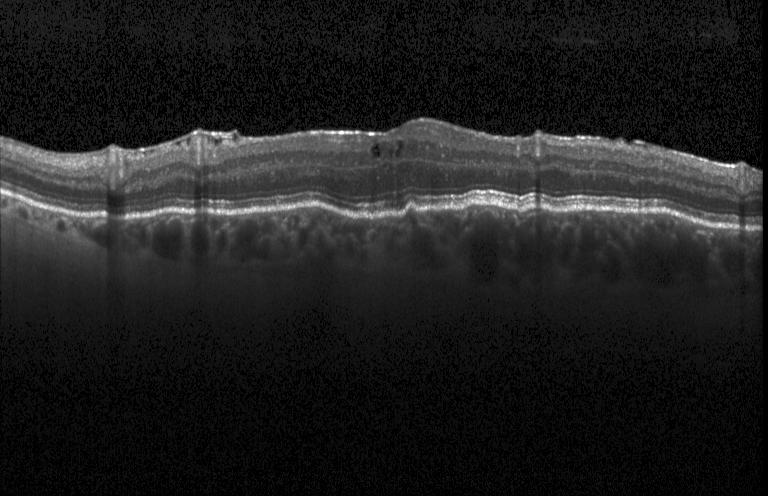

SD-OCT; retinal OCT cross-section — Diagnosis: DME.